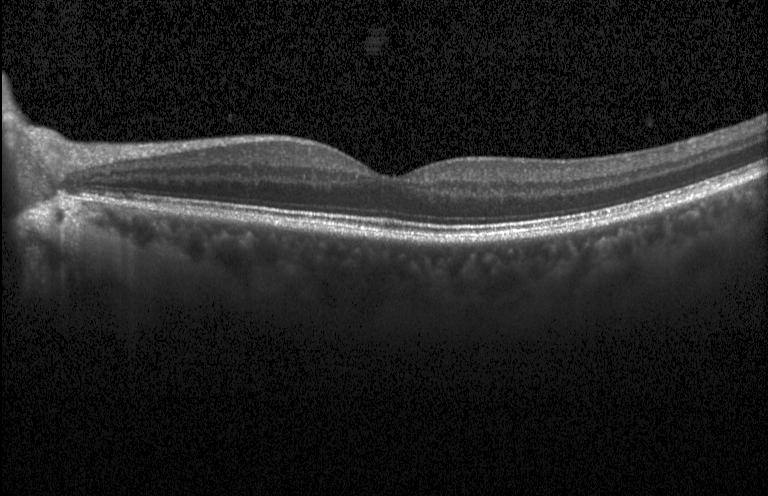

This B-scan demonstrates no choroidal neovascularization, diabetic macular edema, or drusen.